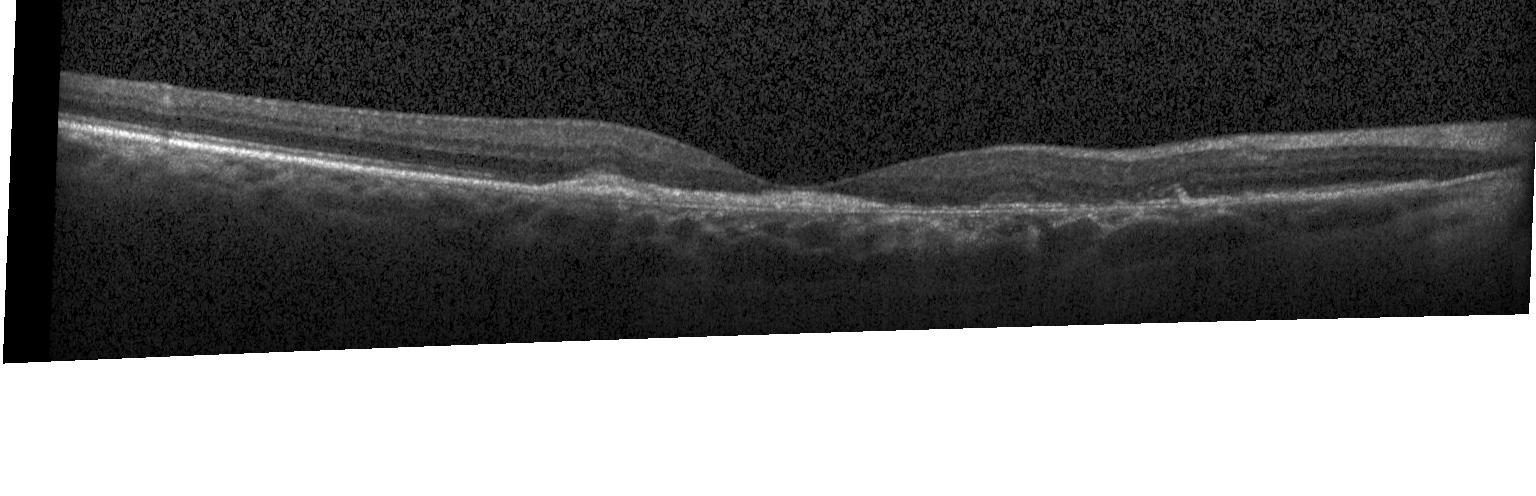

CNV.